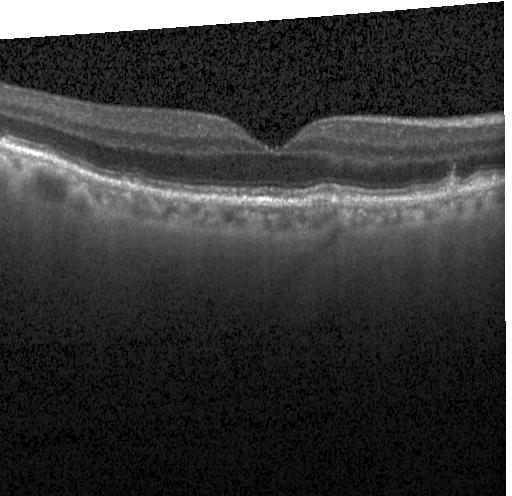

The scan shows drusen.